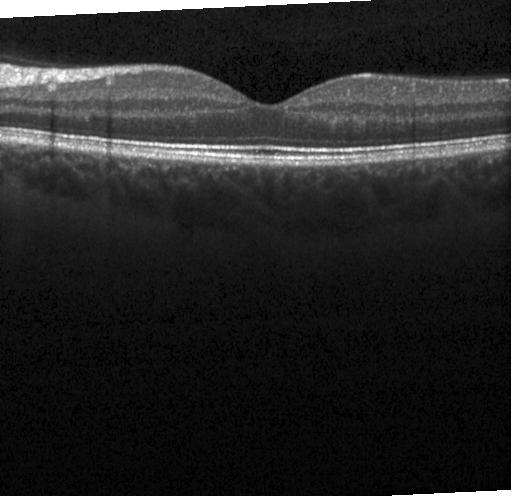 Optical coherence tomography scan — Finding: neither CNV, DME, nor drusen.